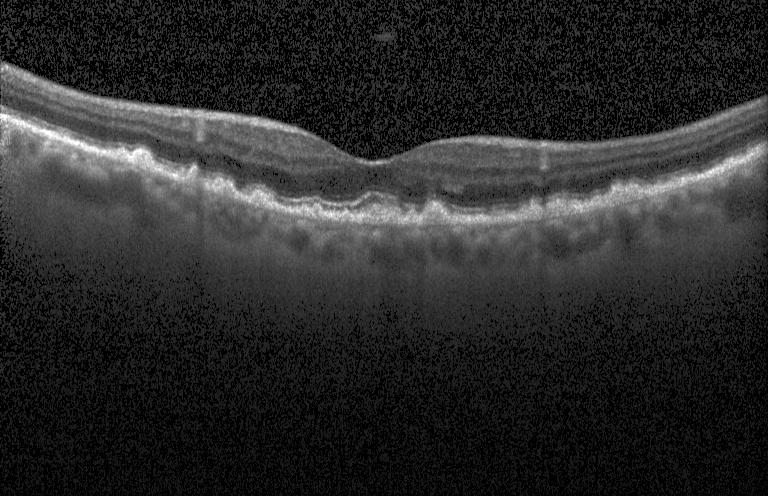 Retinal OCT B-scan. OCT finding: multiple drusen.